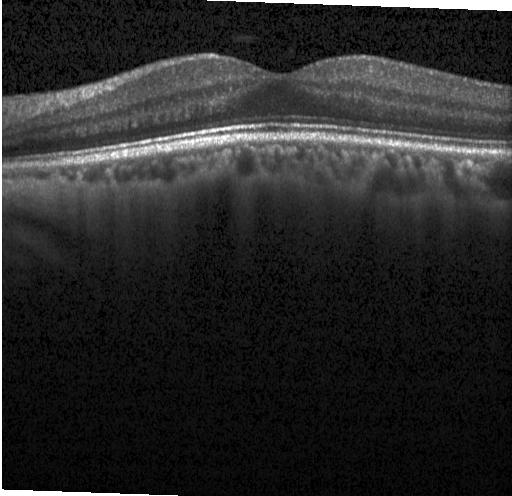
OCT B-scan showing no choroidal neovascularization, diabetic macular edema, or drusen.